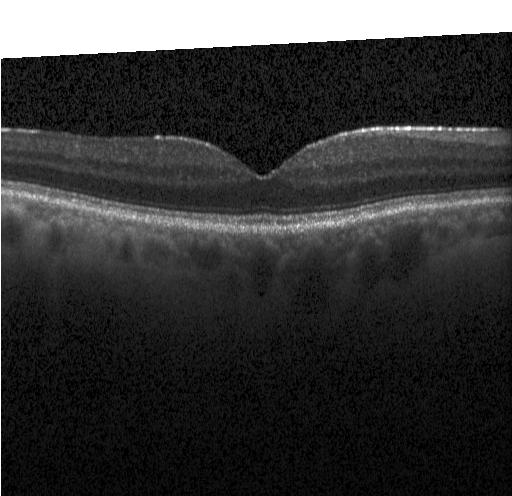 Assessment: no choroidal neovascularization, no diabetic macular edema, and no drusen.